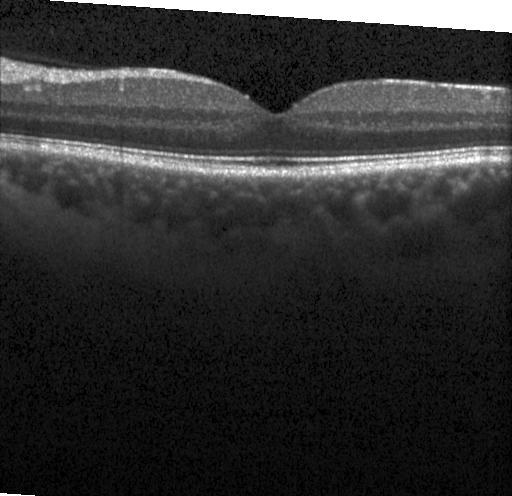
Heidelberg Spectralis. Spectral-domain optical coherence tomography. Retinal OCT cross-section. Horizontal scan through the fovea. This B-scan demonstrates neither CNV, DME, nor drusen.